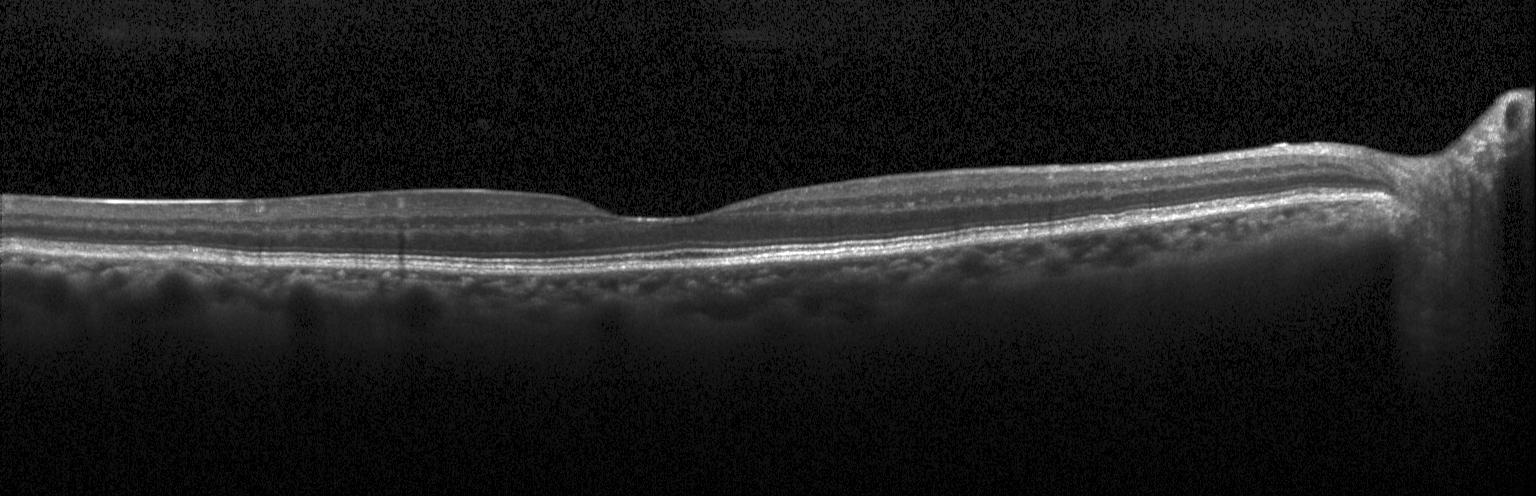 Optical coherence tomography scan.
Diagnosis: neither CNV, DME, nor drusen.